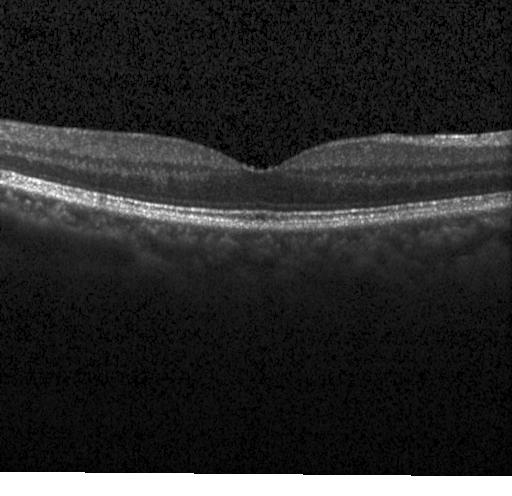 Spectral-domain OCT, centered on the fovea, acquired on a Heidelberg Spectralis, OCT B-scan — Neither CNV, DME, nor drusen.